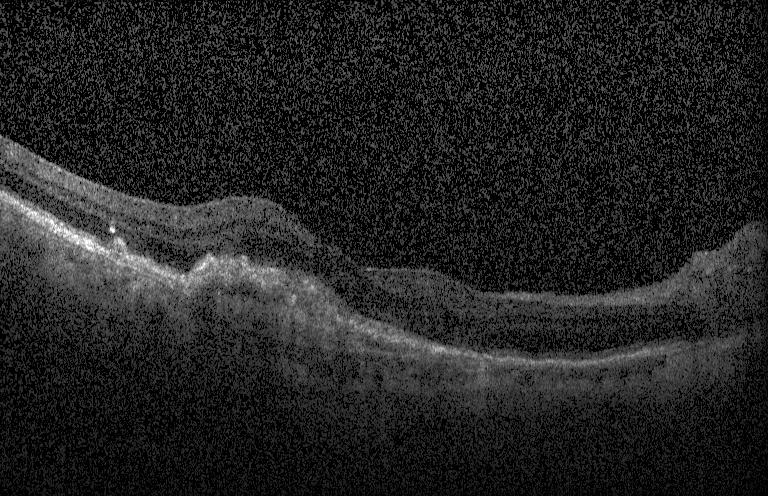 Fovea-centered, spectral-domain optical coherence tomography, retinal OCT cross-section. Macular OCT: choroidal neovascularization (CNV).